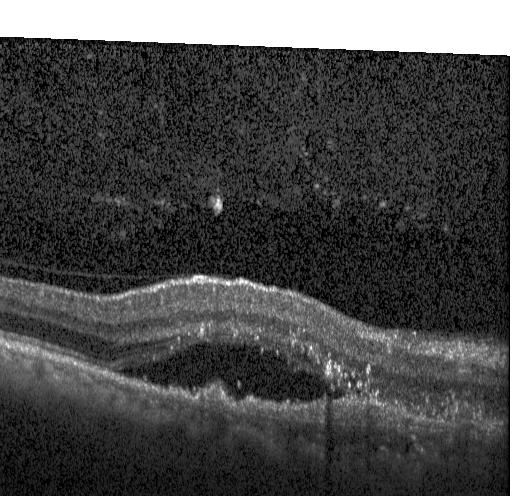 Retinal OCT cross-section showing a choroidal neovascular membrane.